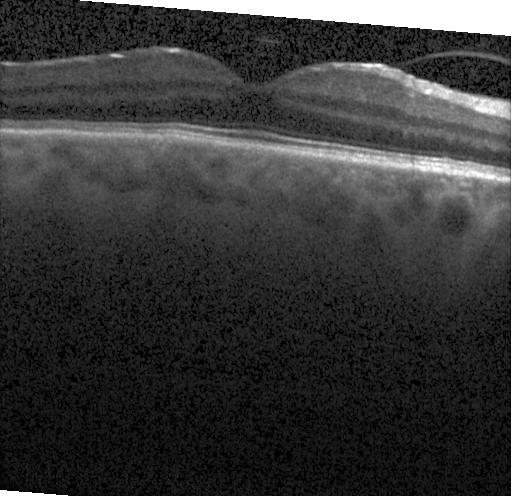

Instrument: Heidelberg Spectralis. SD-OCT. Retinal OCT cross-section. Centered on the fovea
OCT finding: neither choroidal neovascularization, diabetic macular edema, nor drusen.